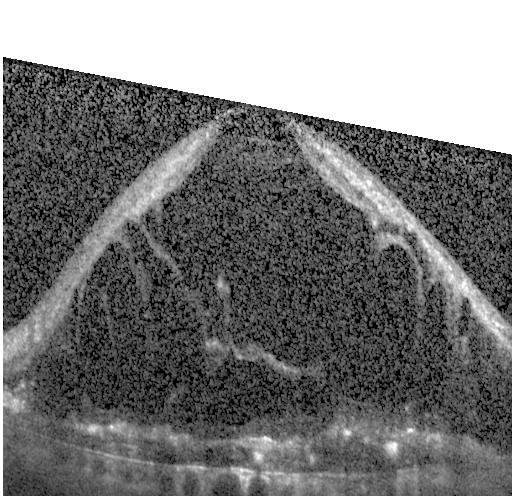
Finding: a choroidal neovascular membrane.